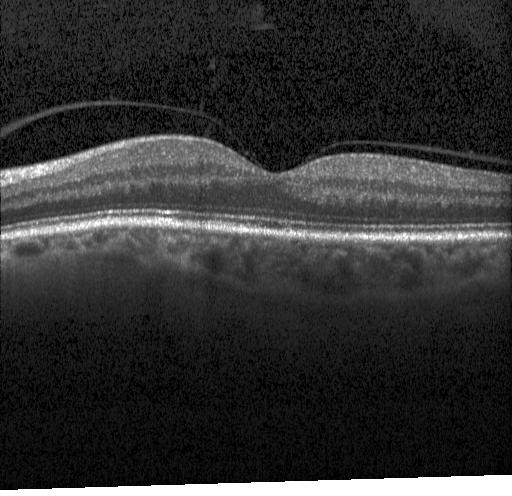
Optical coherence tomography B-scan.
Neither choroidal neovascularization, diabetic macular edema, nor drusen.